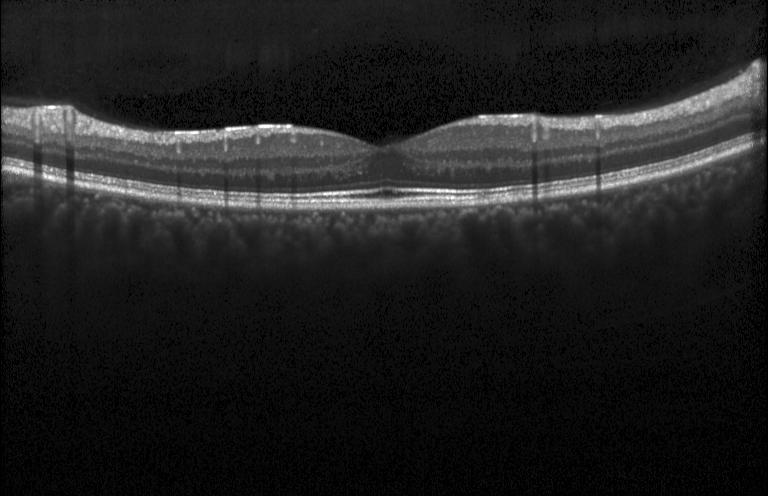
Assessment: neither choroidal neovascularization, diabetic macular edema, nor drusen.